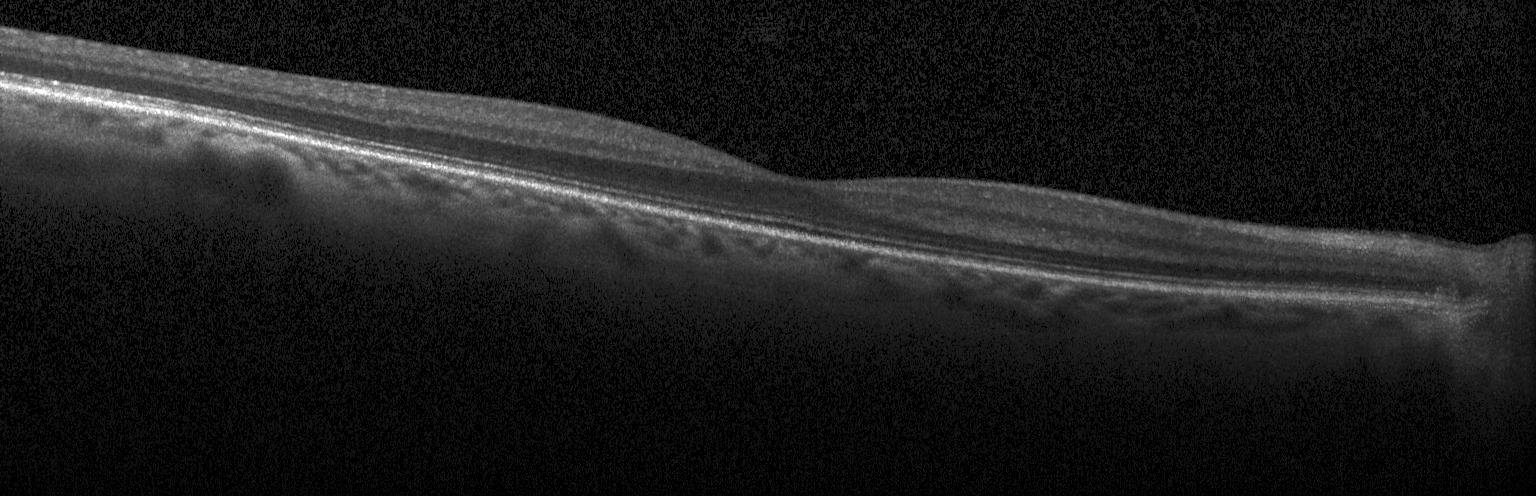 Optical coherence tomography B-scan. Diagnosis: no evidence of choroidal neovascularization, diabetic macular edema, or drusen.